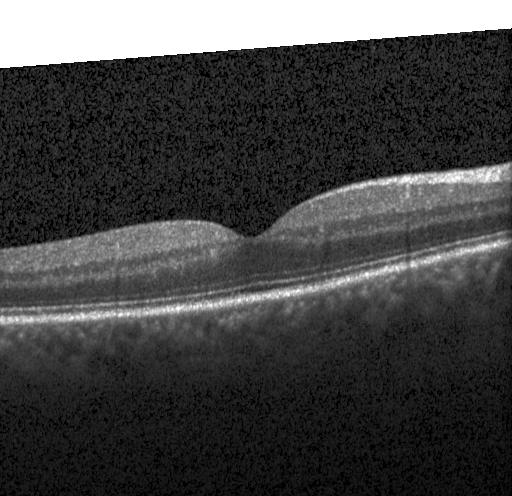
Diagnosis: no evidence of choroidal neovascularization, diabetic macular edema, or drusen.